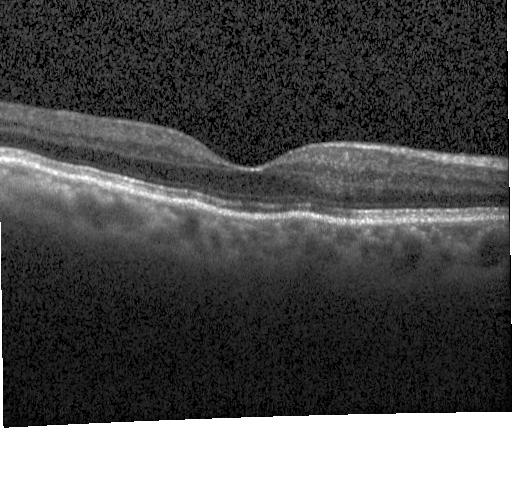 OCT B-scan, spectral-domain OCT, Heidelberg Spectralis OCT system
The scan shows neither choroidal neovascularization, diabetic macular edema, nor drusen.